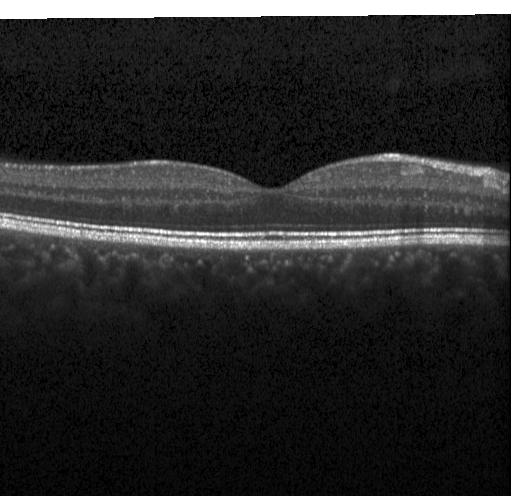
Retinal OCT cross-section
This B-scan demonstrates neither choroidal neovascularization, diabetic macular edema, nor drusen.